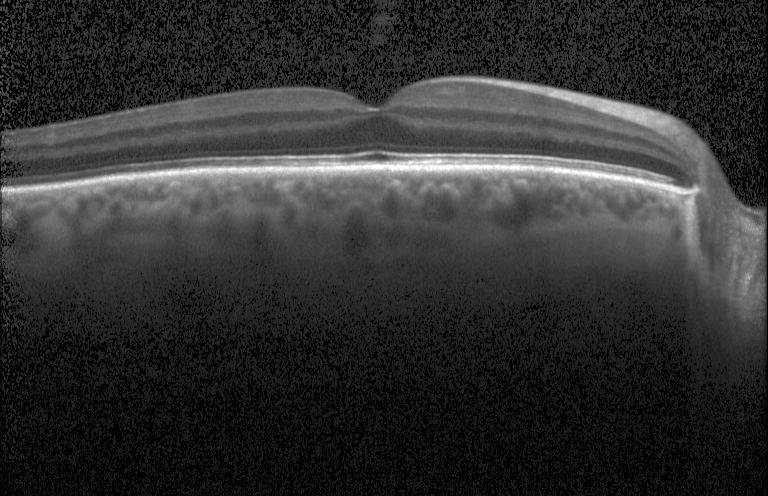 Instrument: Heidelberg Spectralis; through the macula; optical coherence tomography scan; SD-OCT. OCT finding: neither CNV, DME, nor drusen.